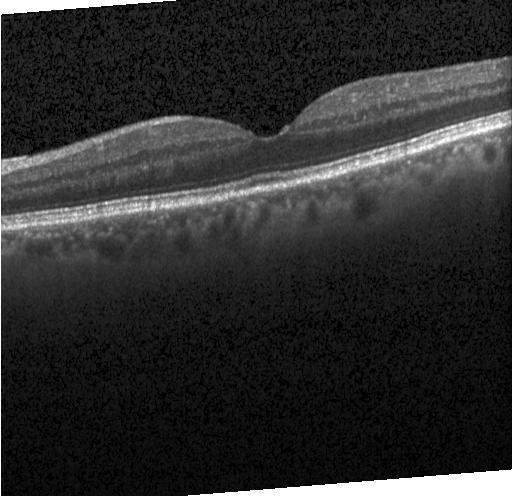 Impression: neither CNV, DME, nor drusen.